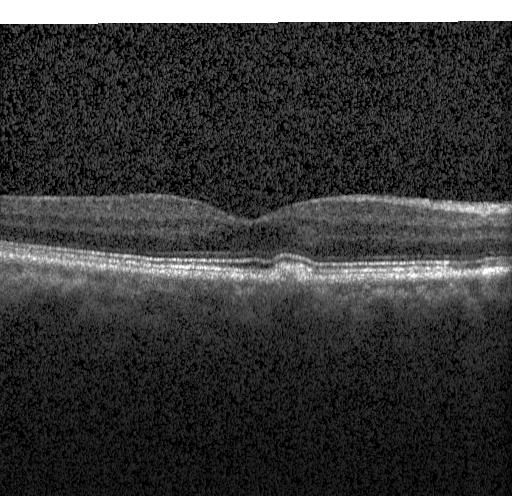 Through the macula; optical coherence tomography scan. The scan shows drusen.